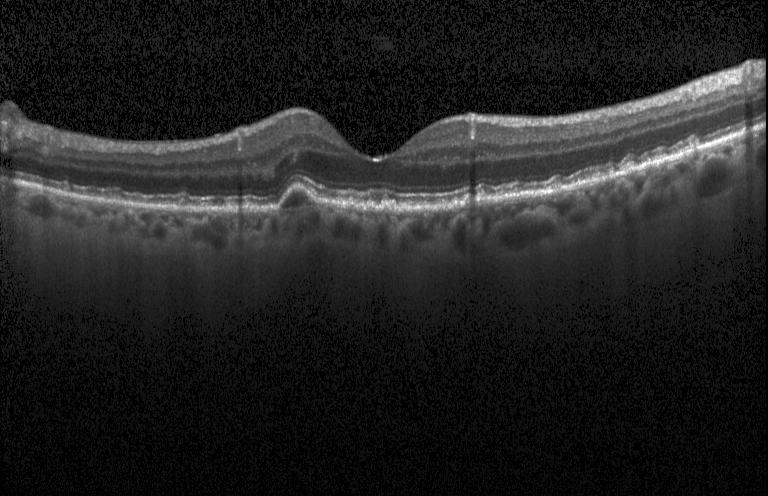

Instrument: Heidelberg Spectralis · optical coherence tomography scan · fovea-centered — This B-scan demonstrates multiple drusen.